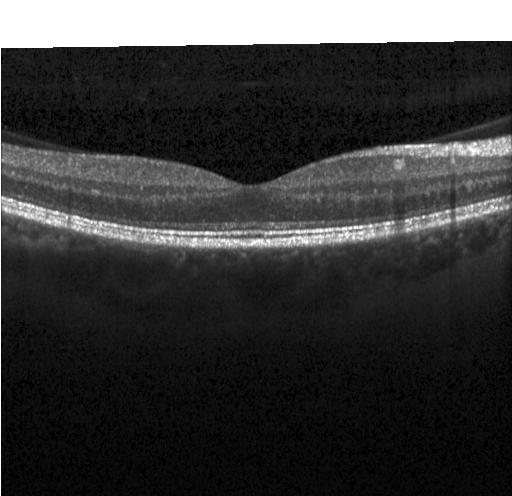
Acquired on a Heidelberg Spectralis, OCT B-scan.
Dx: neither choroidal neovascularization, diabetic macular edema, nor drusen.